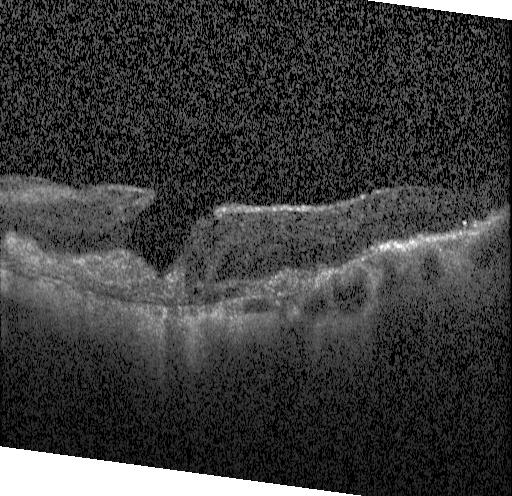
Retinal OCT cross-section
Impression: CNV.